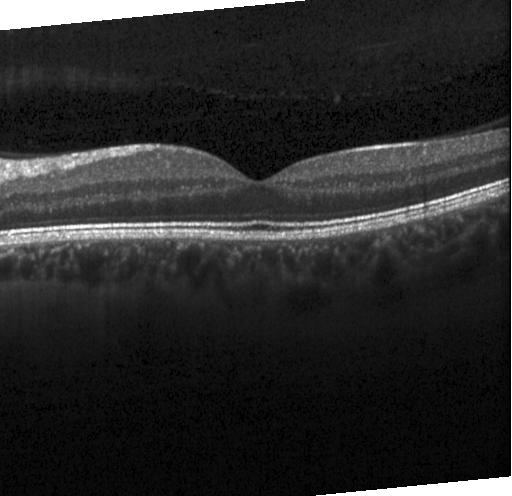 Fovea-centered. Optical coherence tomography B-scan.
The scan shows no CNV, DME, or drusen.